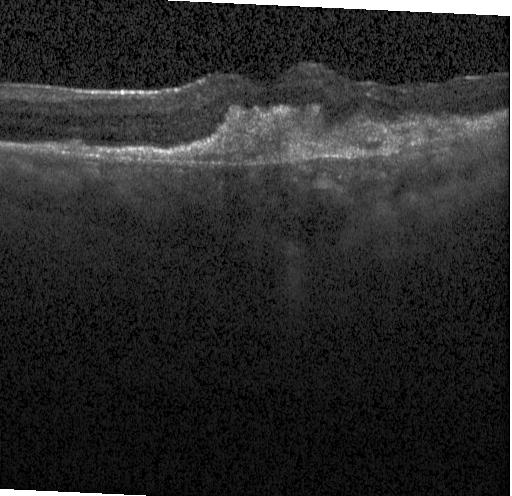 Spectral-domain optical coherence tomography. Through the macula. Optical coherence tomography scan.
Dx: a choroidal neovascular membrane.